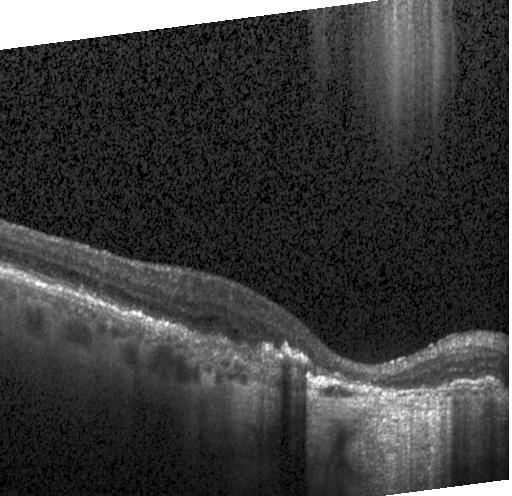

Optical coherence tomography B-scan · horizontal scan through the fovea
Impression: a choroidal neovascular membrane.